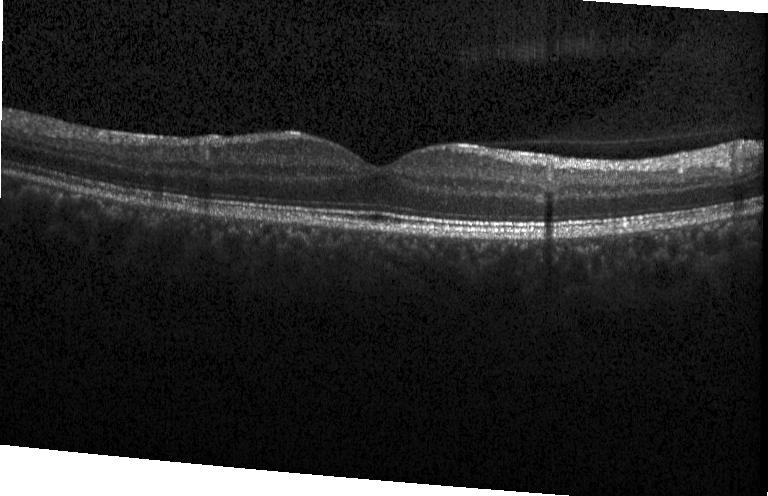

Spectral-domain OCT; optical coherence tomography B-scan — Assessment: no CNV, DME, or drusen.